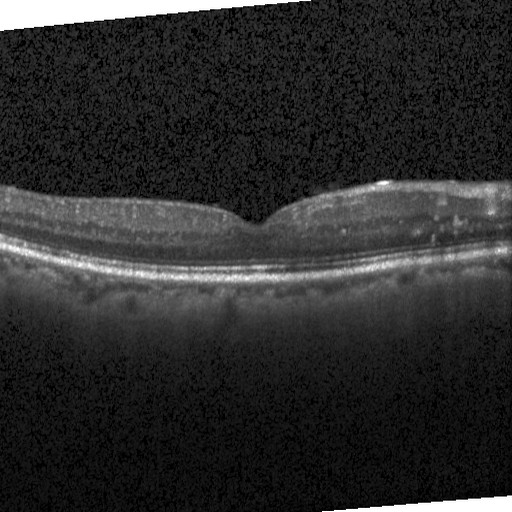

OCT line scan. Through the macula. Heidelberg Spectralis. SD-OCT — Impression: DME.